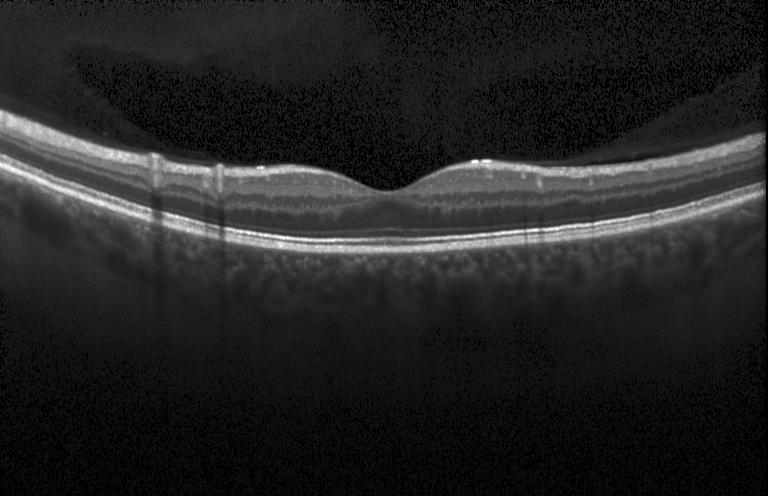
Instrument: Heidelberg Spectralis; OCT B-scan; SD-OCT. Finding: no CNV, no DME, and no drusen.